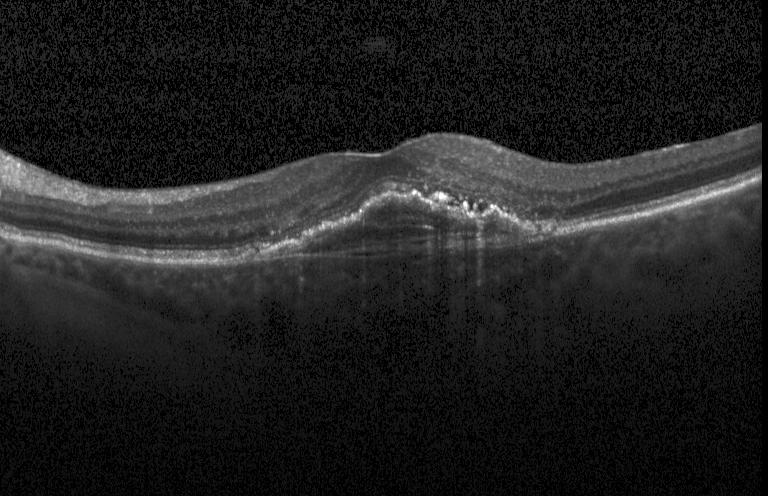
Macular scan; retinal OCT B-scan; spectral-domain OCT; instrument: Heidelberg Spectralis. Impression: a choroidal neovascular membrane.